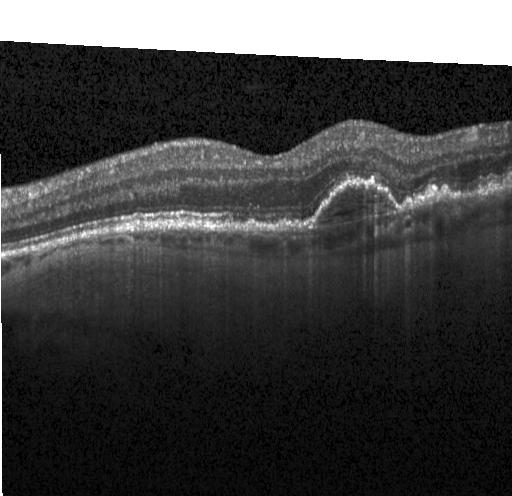
OCT line scan — Diagnosis: a choroidal neovascular membrane.